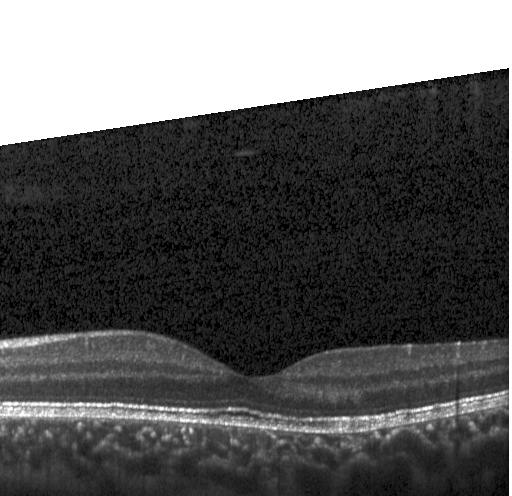 Macular scan · retinal OCT cross-section — Assessment: no choroidal neovascularization, no diabetic macular edema, and no drusen.